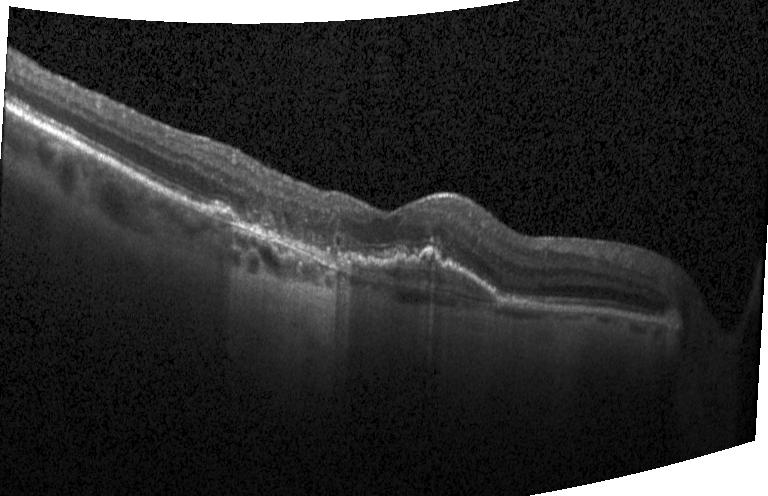 OCT finding: a choroidal neovascular membrane.